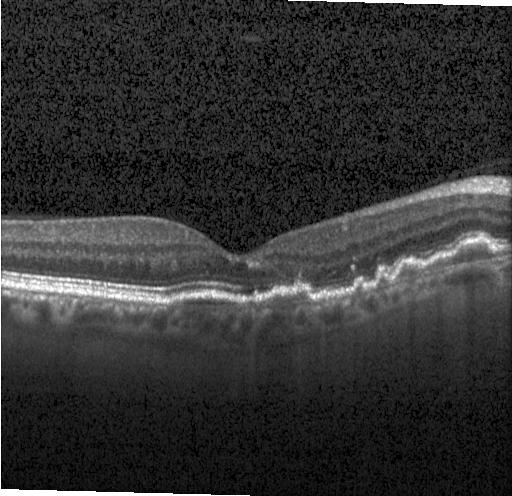 Retinal OCT cross-section showing a choroidal neovascular membrane.